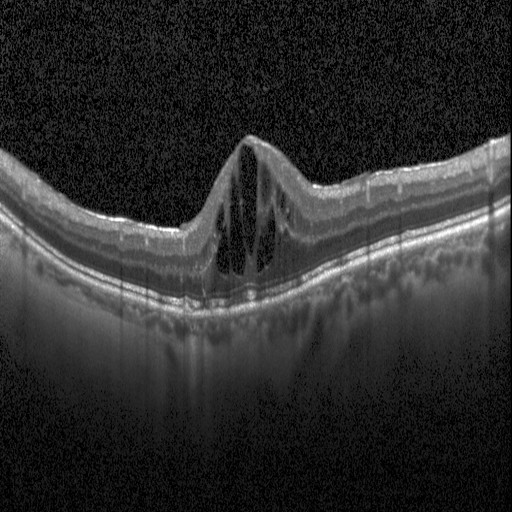
Dx: diabetic macular edema.